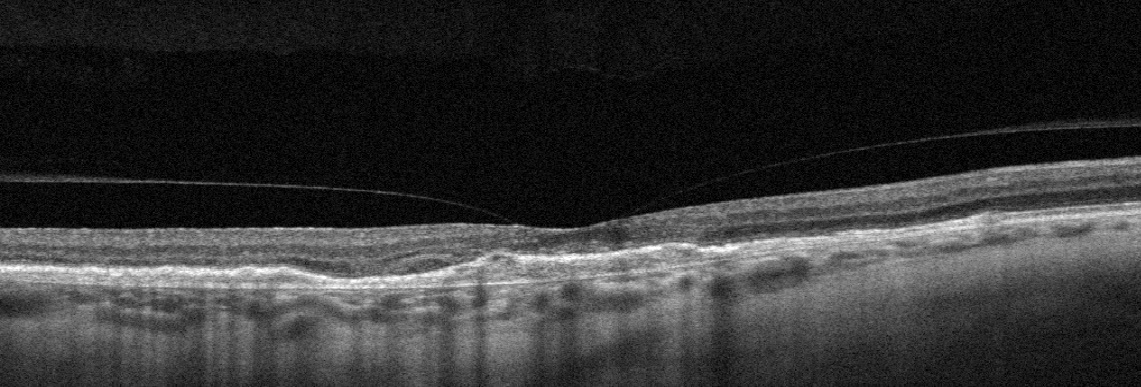

OCT line scan, macular scan — The scan shows age-related macular degeneration (AMD).